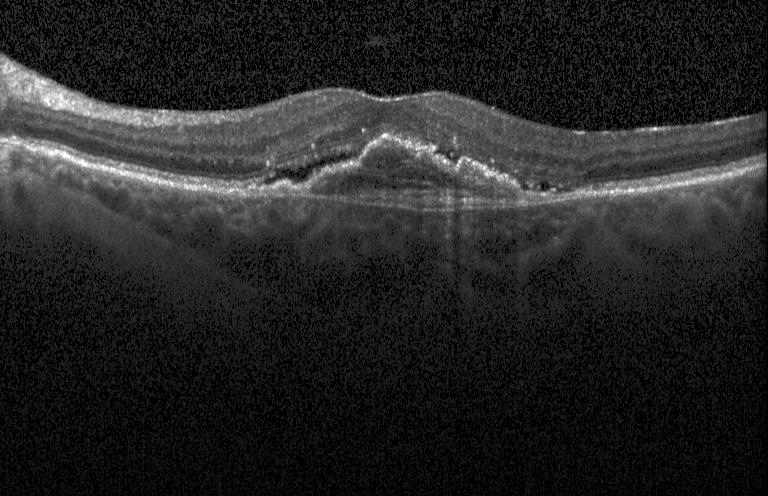

Macular OCT: CNV.